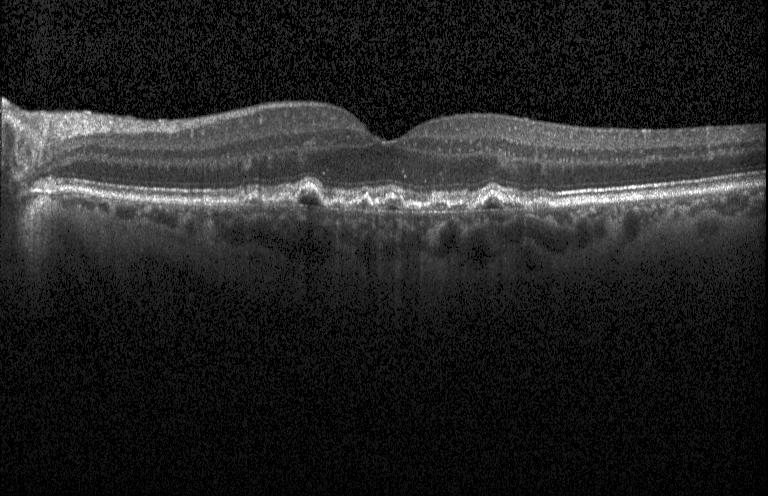
Macular scan. Optical coherence tomography scan.
Macular OCT: multiple drusen.